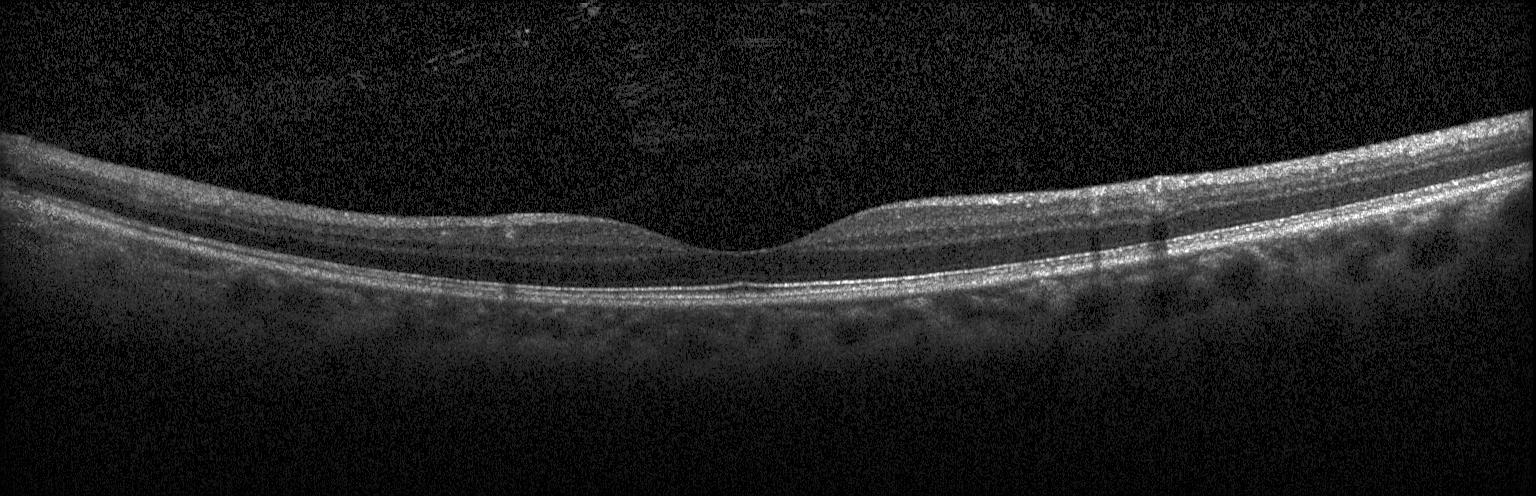

Retinal OCT B-scan.
Diagnosis: neither CNV, DME, nor drusen.